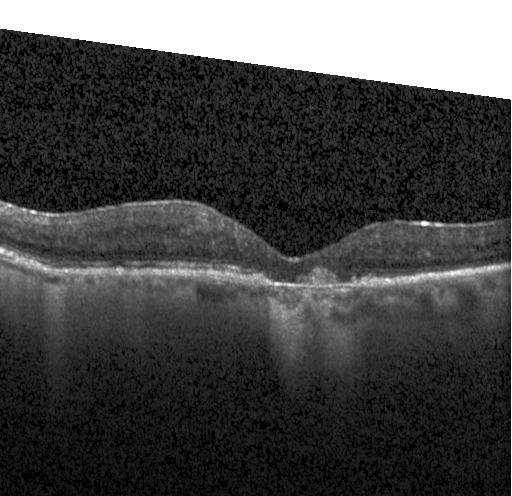
OCT scan showing a choroidal neovascular membrane.